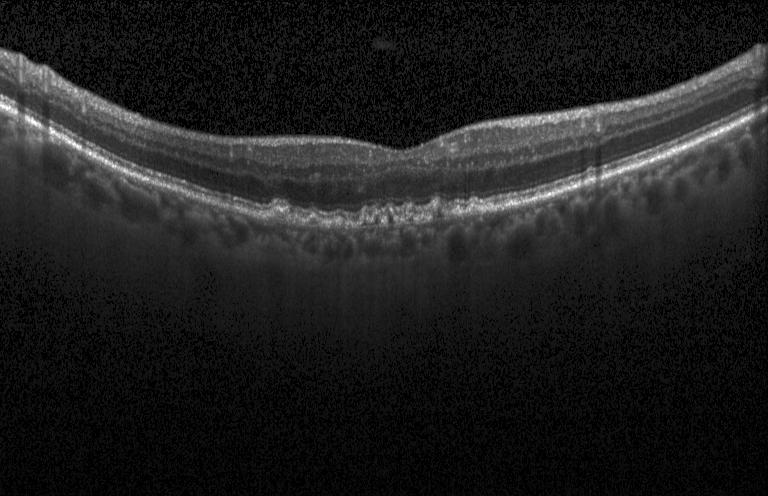
Retinal OCT B-scan — Diagnosis: multiple drusen.